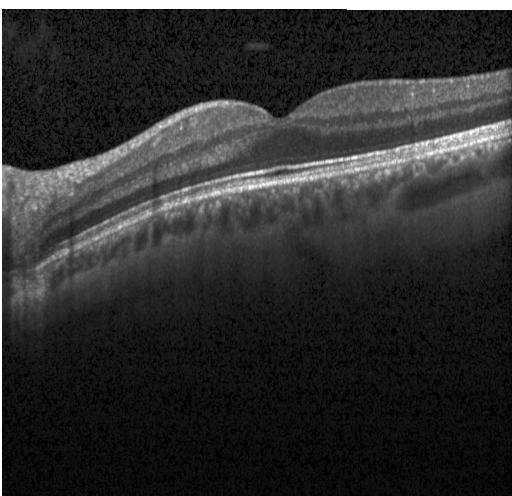 Spectral-domain OCT B-scan: neither choroidal neovascularization, diabetic macular edema, nor drusen.